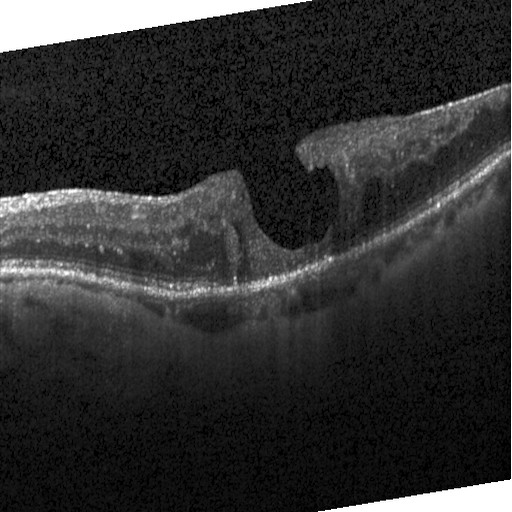 Diabetic macular edema (DME).